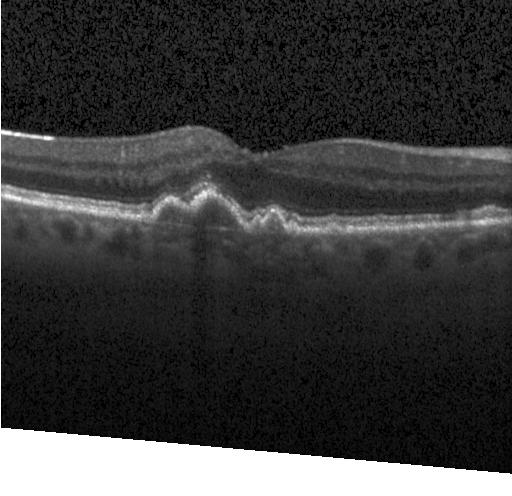 Assessment: sub-RPE drusenoid deposits.